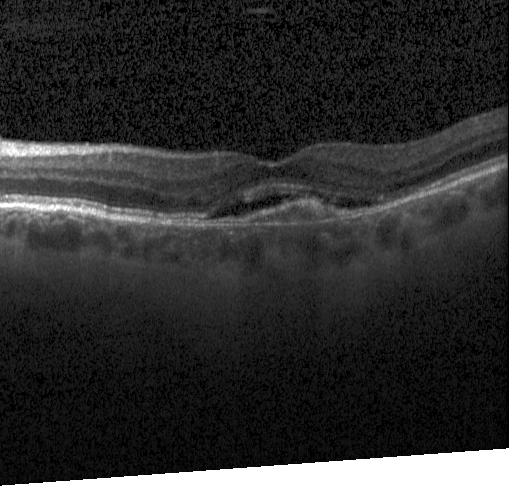
Acquired on a Heidelberg Spectralis, retinal OCT B-scan
Assessment: a choroidal neovascular membrane.